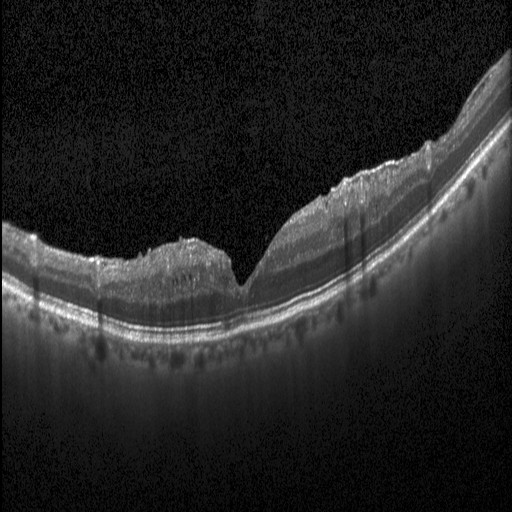

Retinal OCT cross-section showing diabetic macular edema (DME).